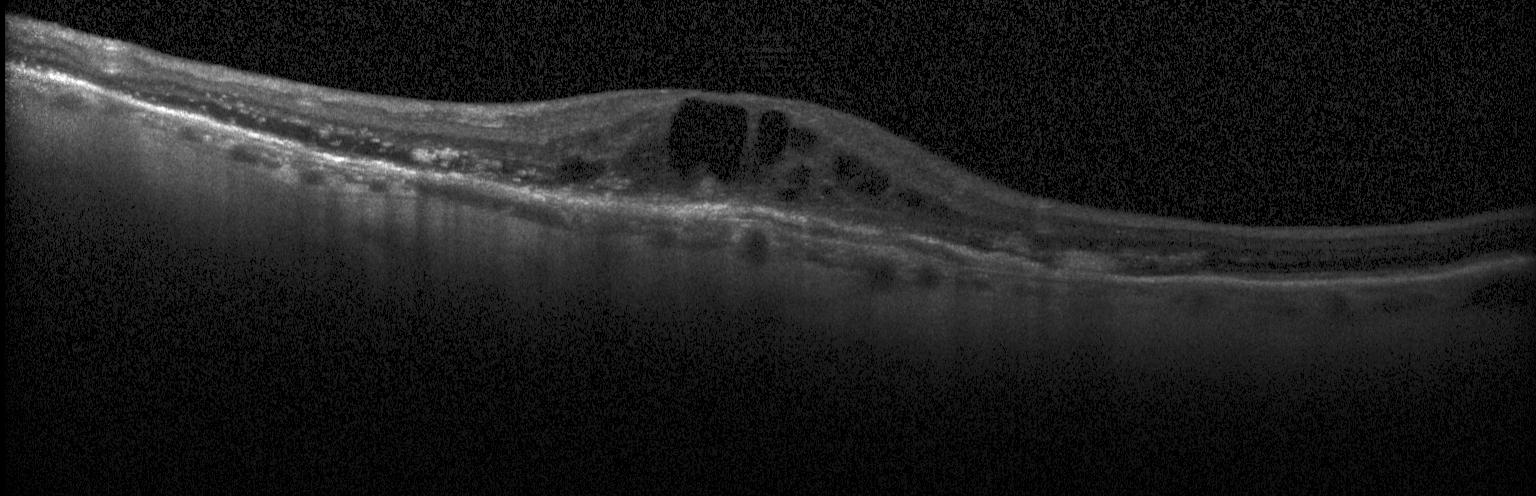

OCT B-scan showing CNV.